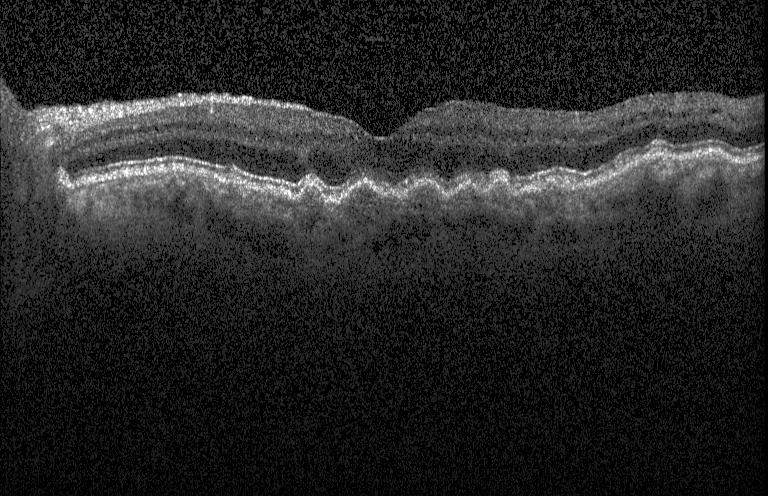
Drusen.